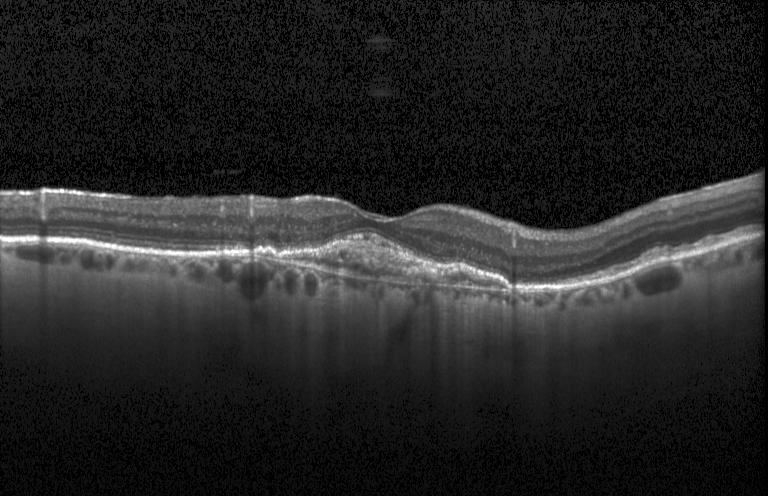
This B-scan demonstrates choroidal neovascularization (CNV).